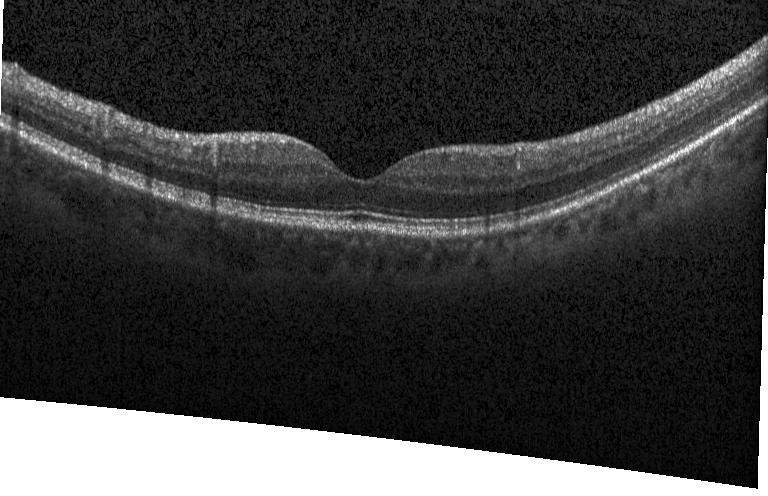
Spectral-domain OCT B-scan: no CNV, no DME, and no drusen.